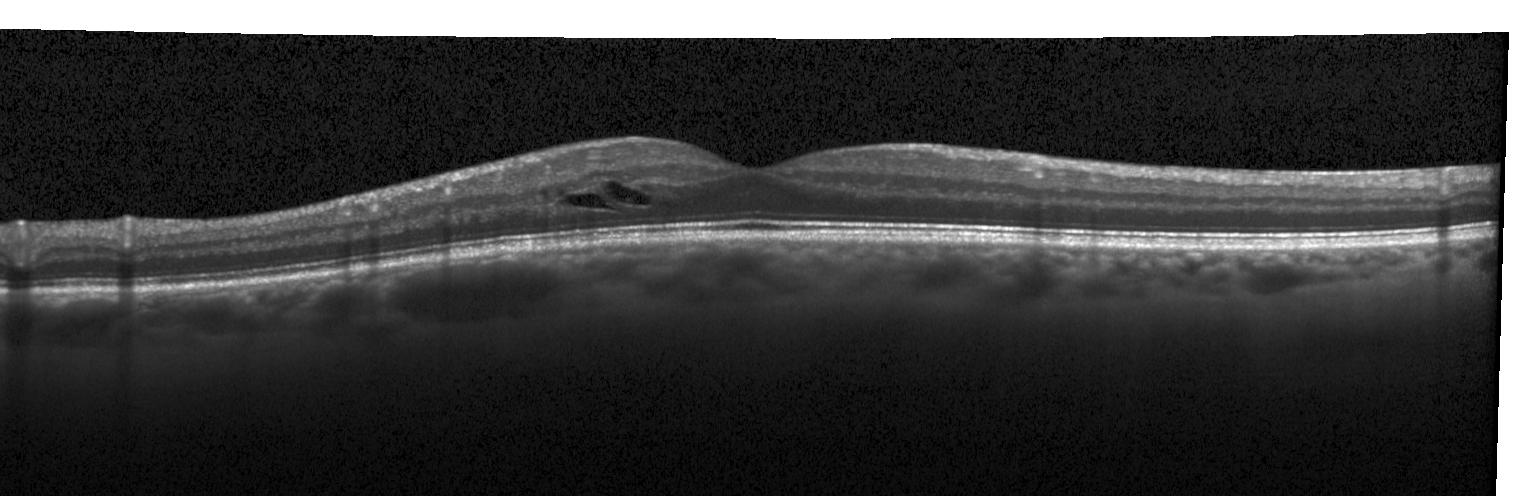
Finding: DME.